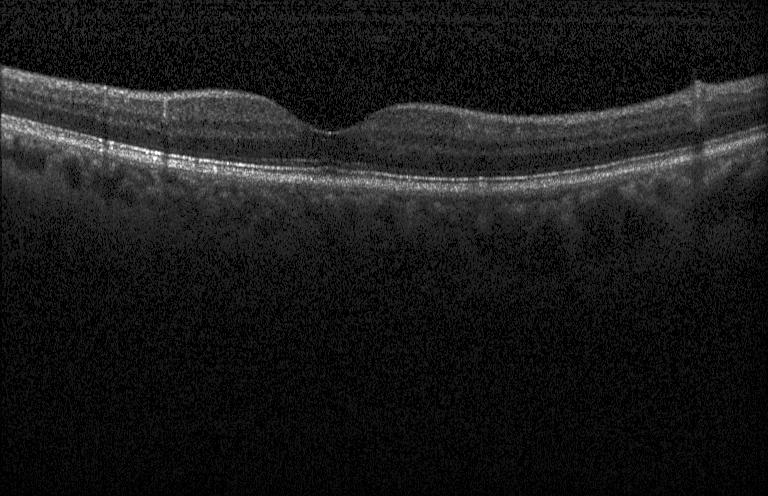

Impression: no choroidal neovascularization, no diabetic macular edema, and no drusen.